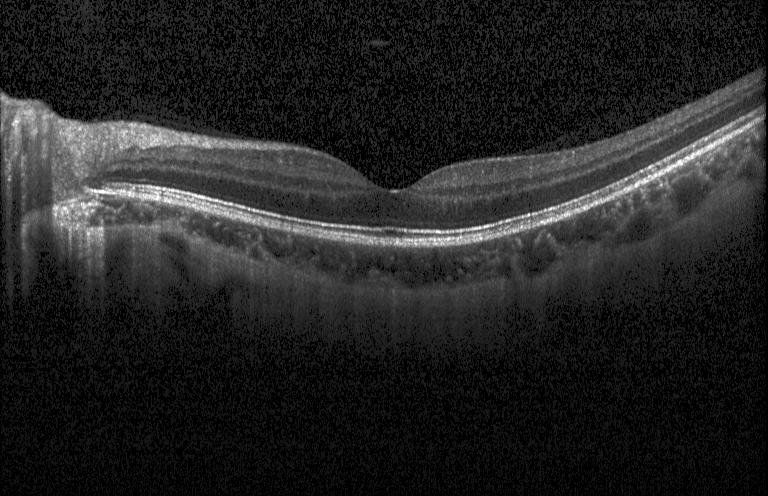

Retinal OCT cross-section. SD-OCT. Macular scan — Impression: no choroidal neovascularization, no diabetic macular edema, and no drusen.